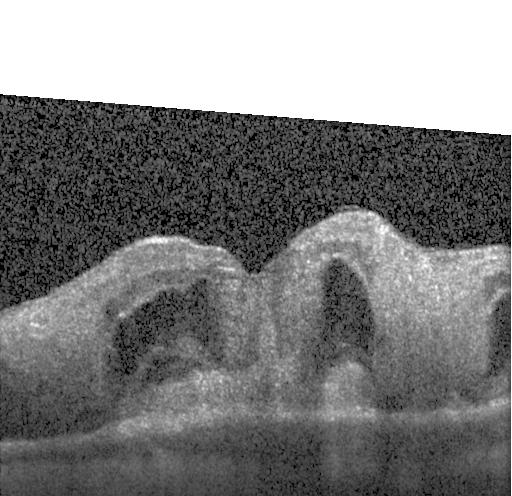 OCT scan showing a choroidal neovascular membrane.